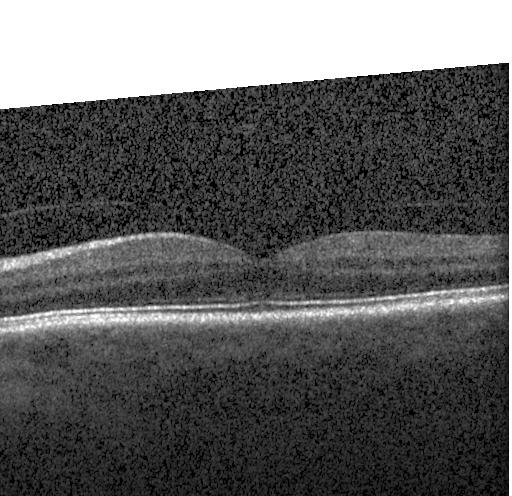
Centered on the fovea, optical coherence tomography scan, acquired on a Heidelberg Spectralis, spectral-domain OCT
Dx: no choroidal neovascularization, diabetic macular edema, or drusen.